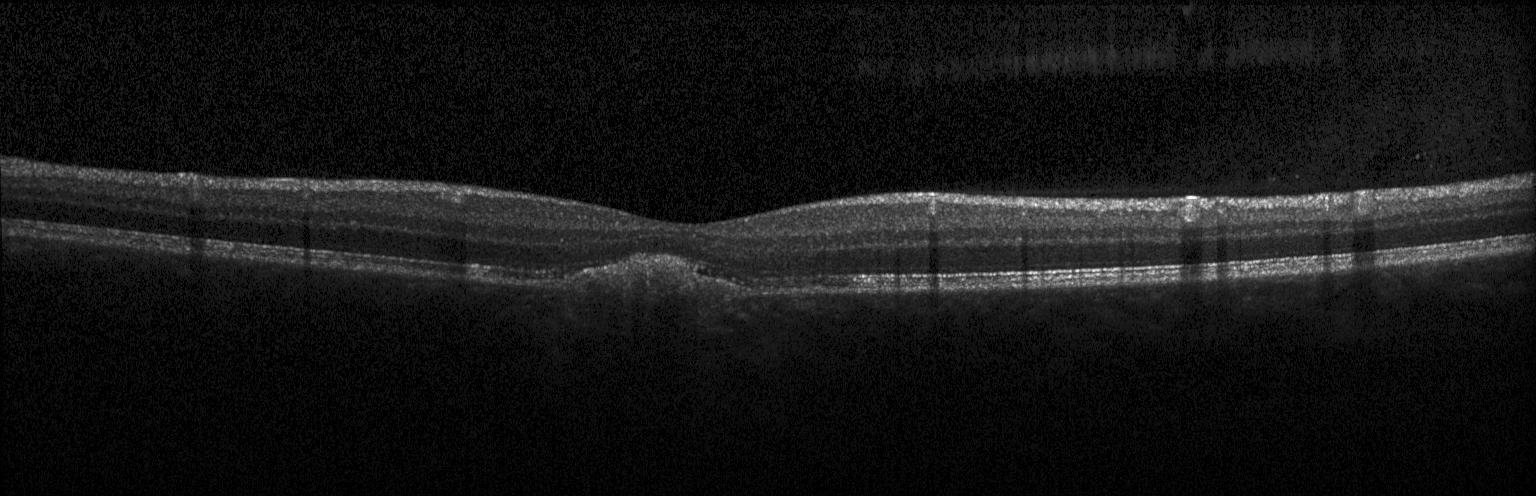

Diagnosis: choroidal neovascularization.